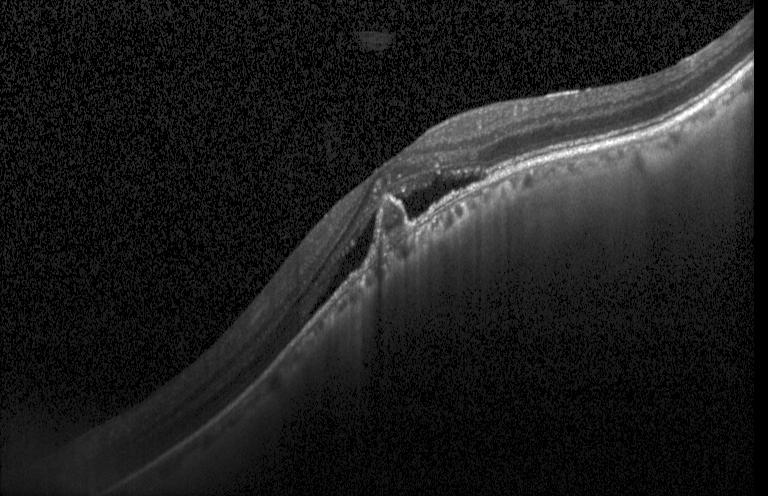 Macular OCT: CNV.